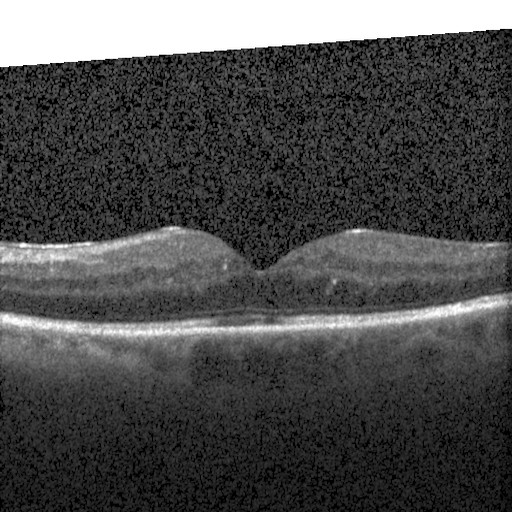

Optical coherence tomography B-scan. DME.